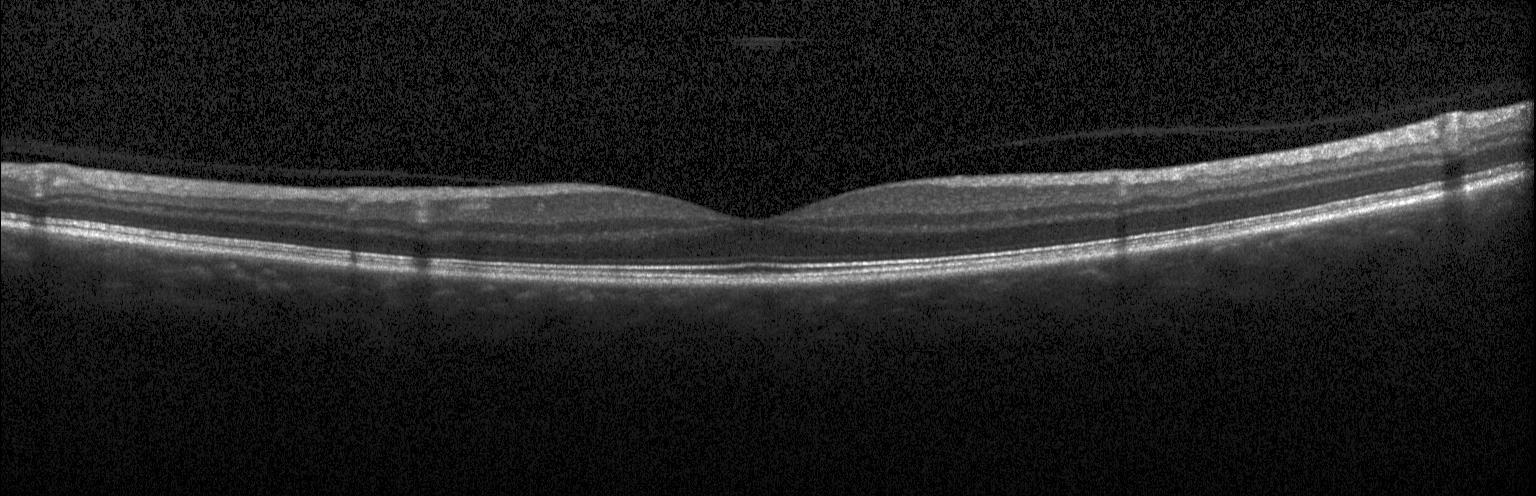 OCT finding: no choroidal neovascularization, no diabetic macular edema, and no drusen.